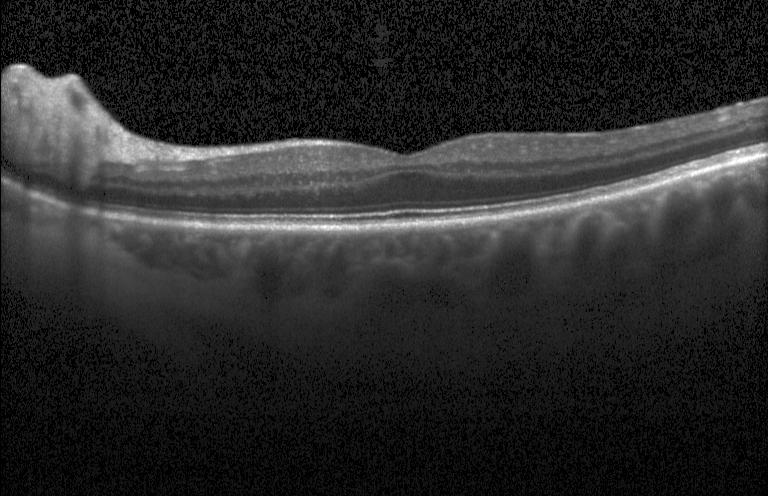 OCT B-scan · Heidelberg Spectralis OCT system · spectral-domain OCT.
Dx: no choroidal neovascularization, no diabetic macular edema, and no drusen.